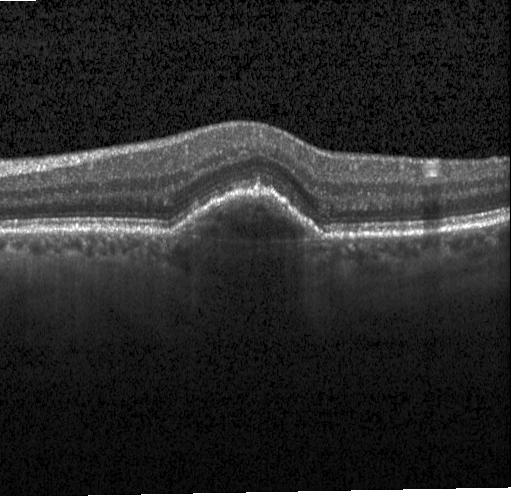
Impression: choroidal neovascularization.